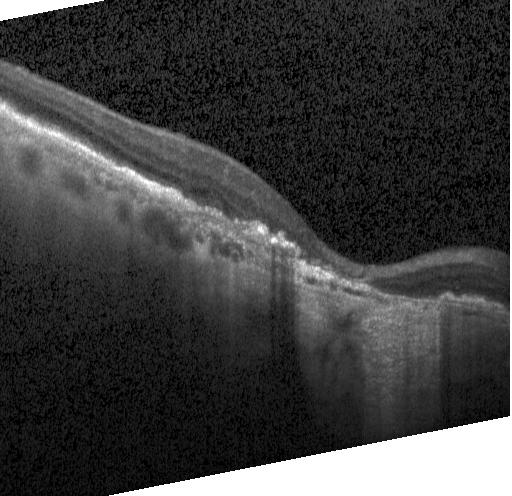
Optical coherence tomography B-scan, Heidelberg Spectralis OCT system, fovea-centered
CNV.